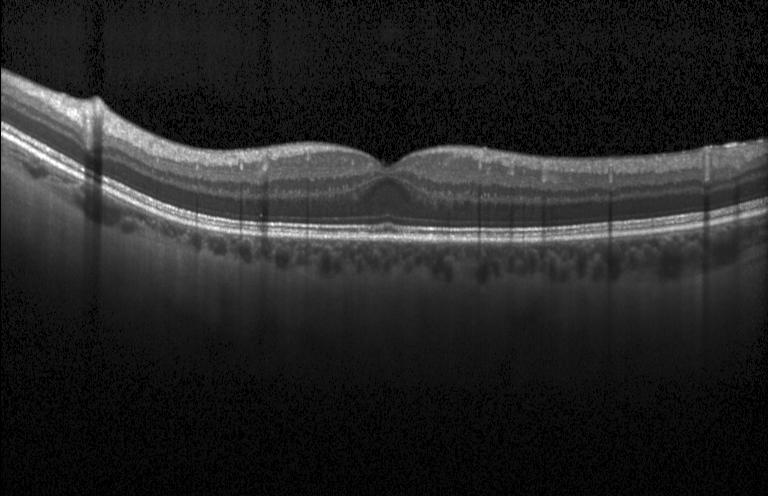 Impression: no choroidal neovascularization, diabetic macular edema, or drusen.